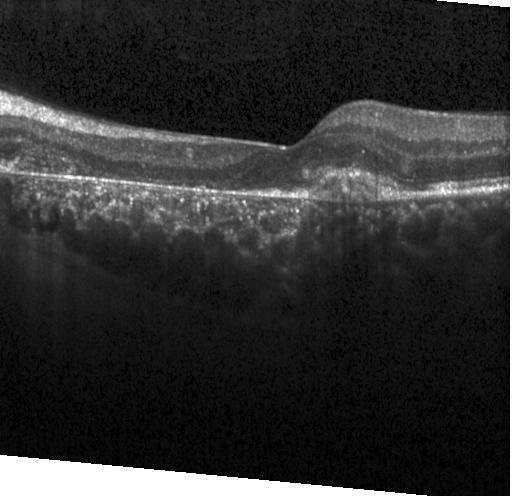
Heidelberg Spectralis OCT system · macular scan · SD-OCT · OCT B-scan — Choroidal neovascularization (CNV).